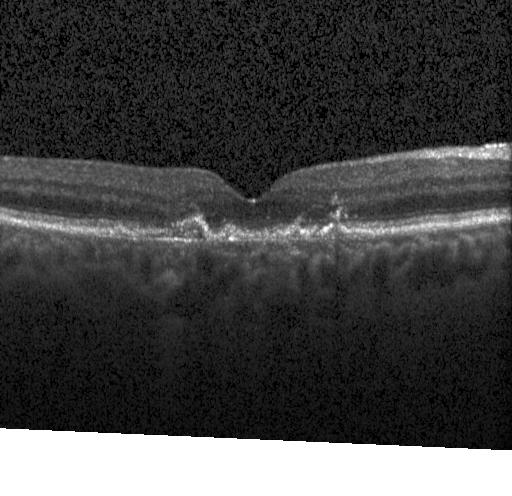

OCT B-scan.
OCT finding: a choroidal neovascular membrane.